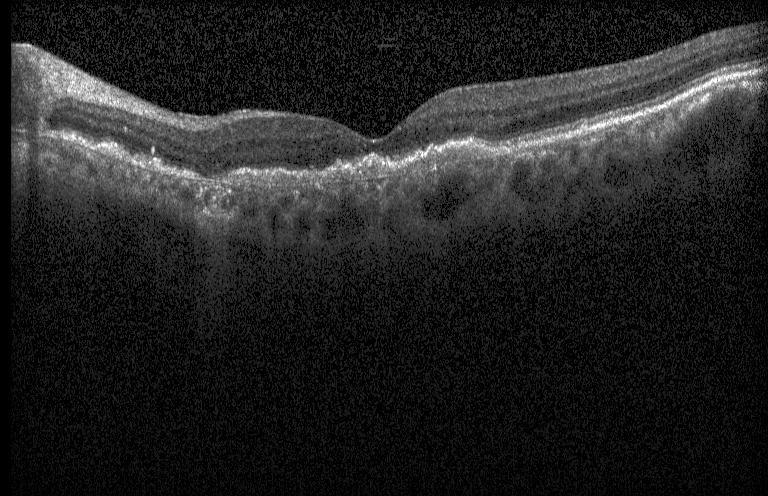 OCT B-scan showing choroidal neovascularization (CNV).